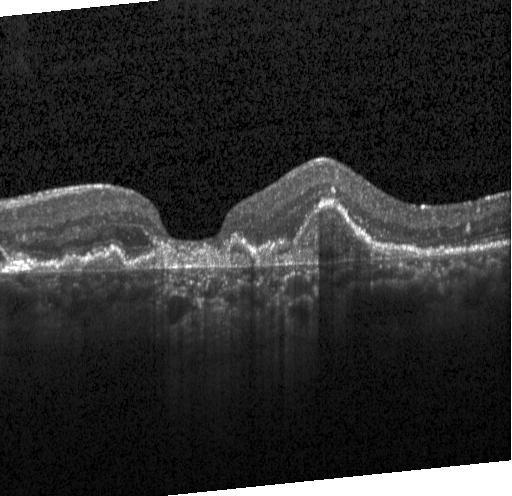
Assessment: choroidal neovascularization.